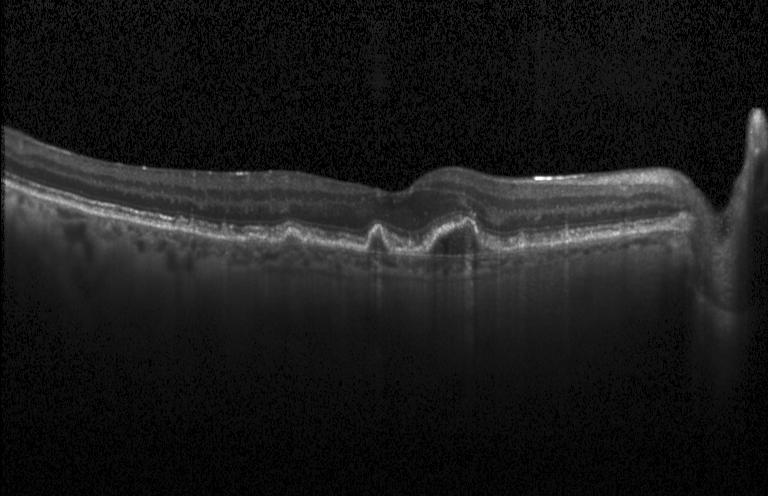 Acquired on a Heidelberg Spectralis; OCT B-scan; SD-OCT; through the macula.
This B-scan demonstrates a choroidal neovascular membrane.